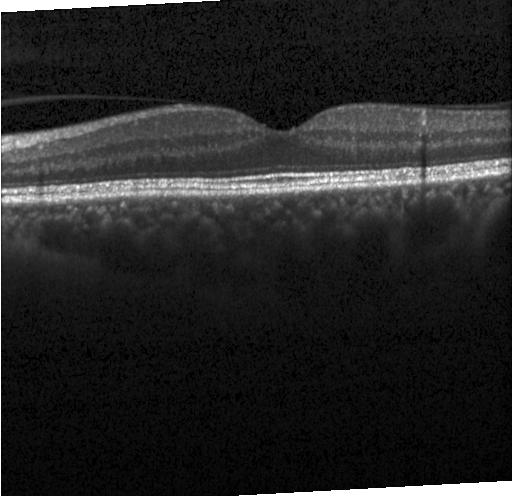

Optical coherence tomography scan. Macular scan. Heidelberg Spectralis OCT system.
Dx: neither CNV, DME, nor drusen.